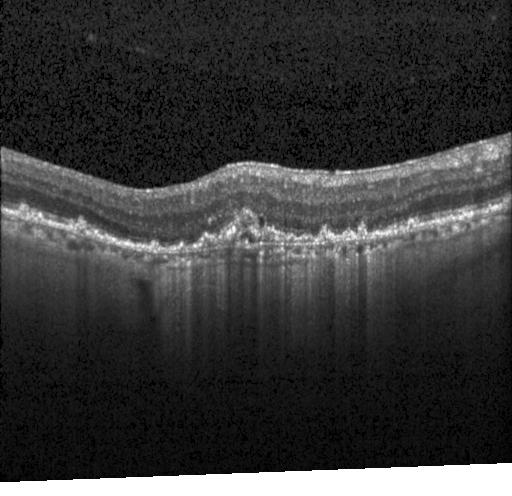

Impression: choroidal neovascularization.